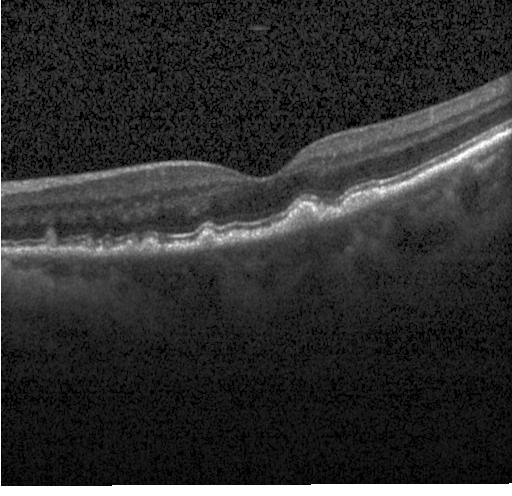 Diagnosis: multiple drusen.